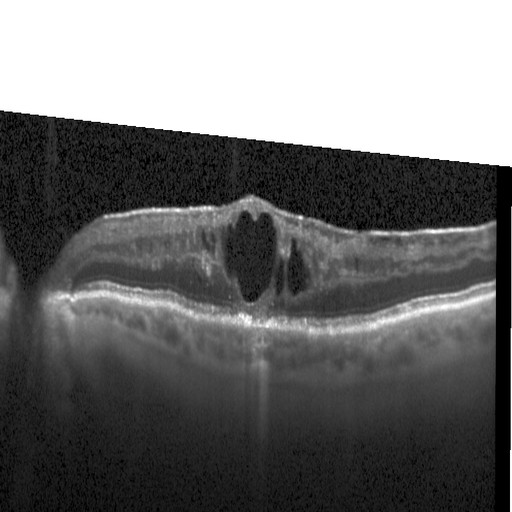 Retinal OCT B-scan, fovea-centered, SD-OCT.
Diabetic macular edema (DME).